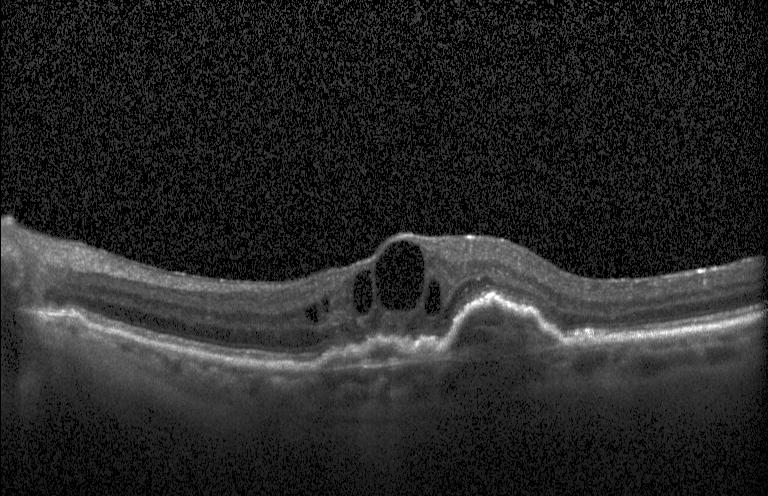 Finding: CNV.